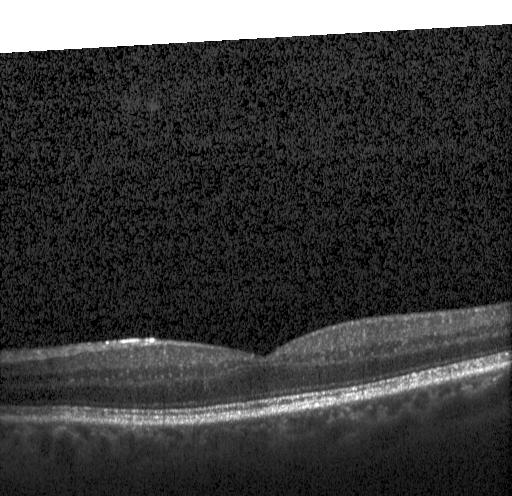 Diagnosis: neither choroidal neovascularization, diabetic macular edema, nor drusen.